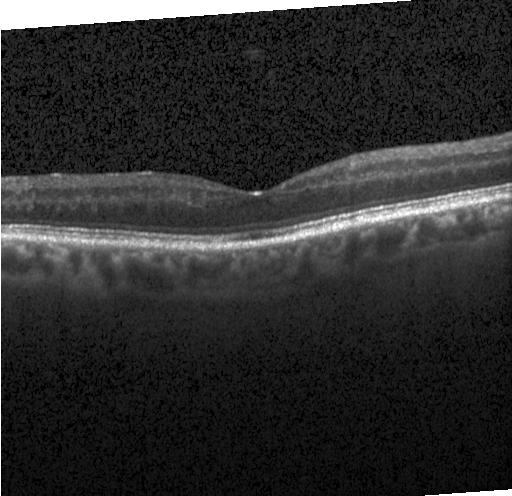 OCT B-scan showing neither choroidal neovascularization, diabetic macular edema, nor drusen.